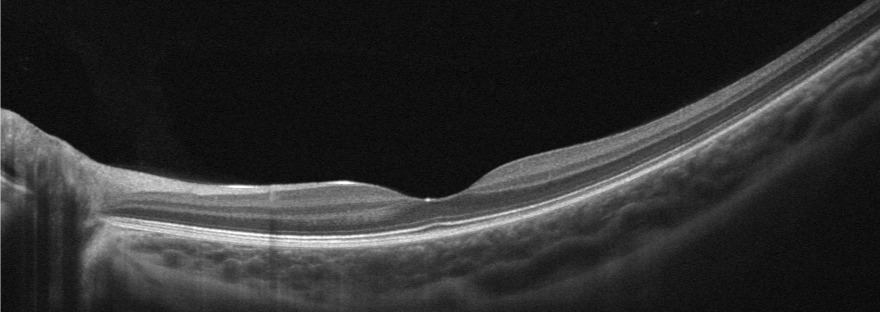

Assessment: no evidence of AMD, DME, ERM, RAO, RVO, or VID.